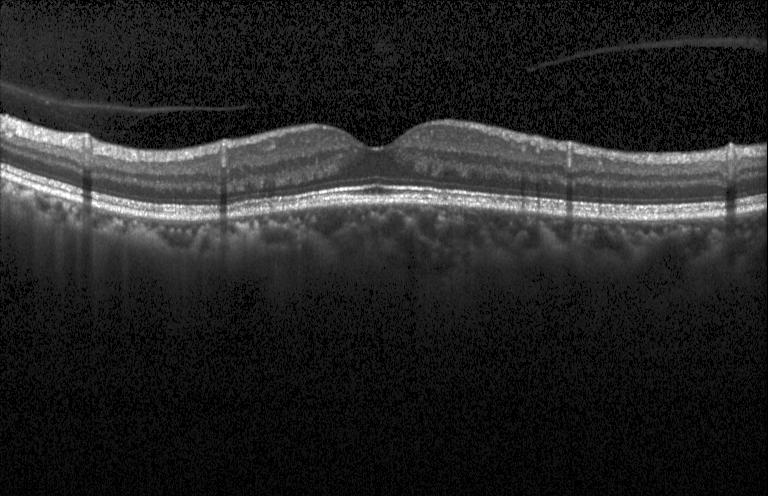

Retinal OCT B-scan, spectral-domain OCT, centered on the fovea. Dx: no evidence of choroidal neovascularization, diabetic macular edema, or drusen.